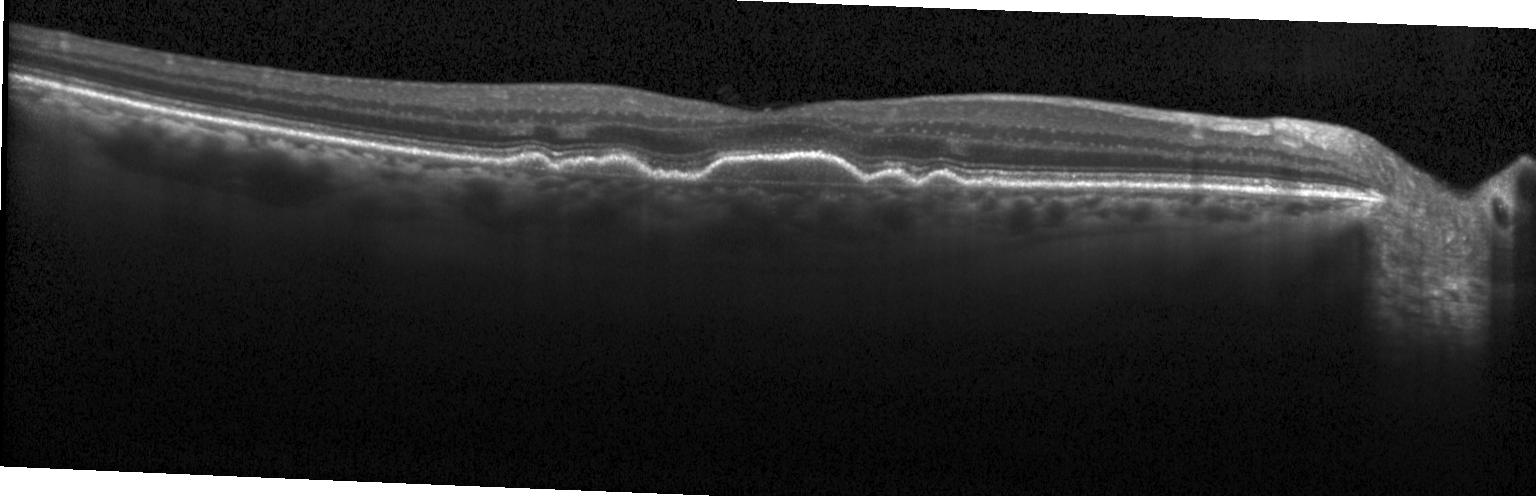 Acquired on a Heidelberg Spectralis, OCT B-scan, spectral-domain optical coherence tomography.
The scan shows choroidal neovascularization.